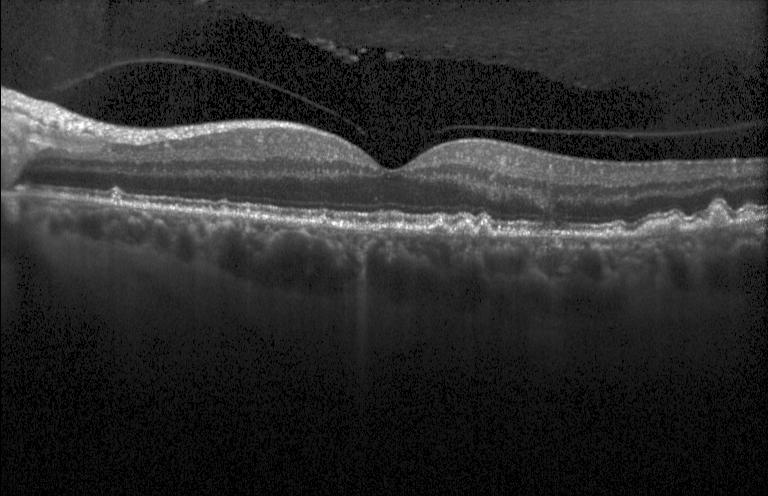
SD-OCT; optical coherence tomography scan.
Finding: drusen.